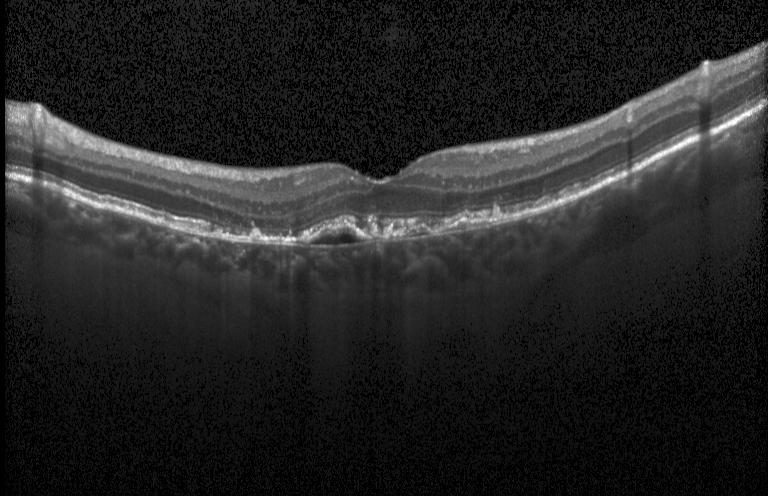 A choroidal neovascular membrane.